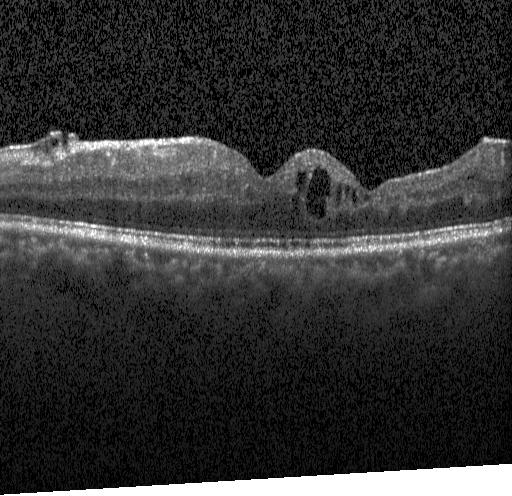 Retinal OCT B-scan — Impression: diabetic macular edema (DME).